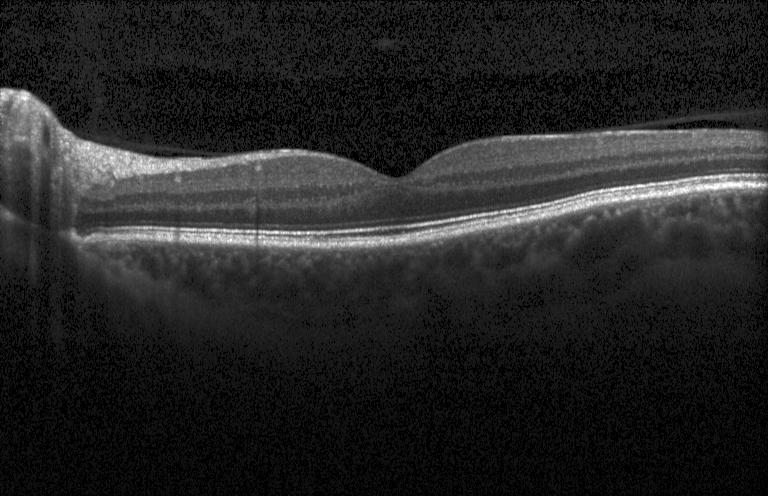

Dx: no choroidal neovascularization, no diabetic macular edema, and no drusen.